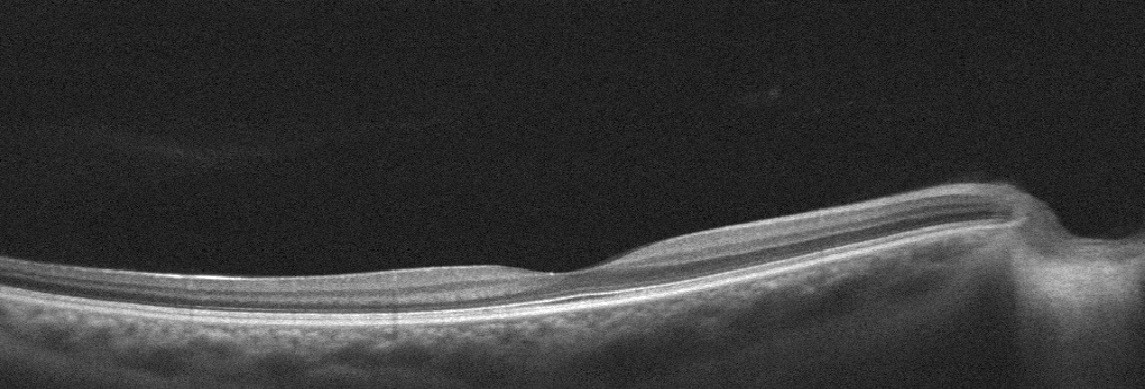 Finding: no AMD, DME, ERM, RAO, RVO, or VID.